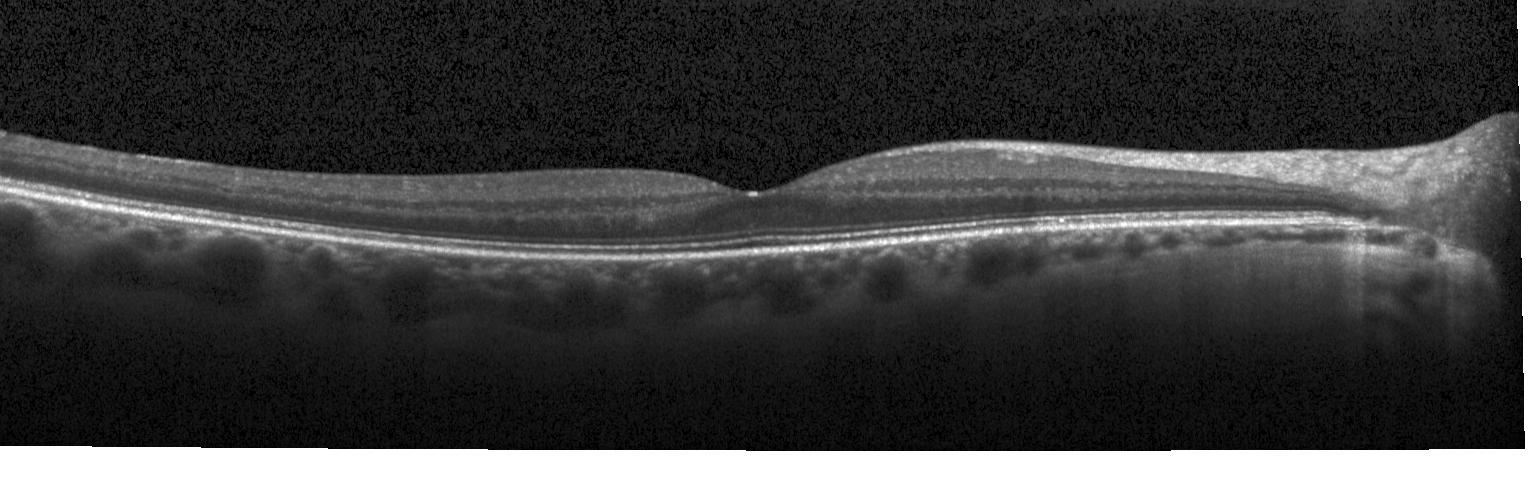

OCT B-scan
Impression: no CNV, no DME, and no drusen.